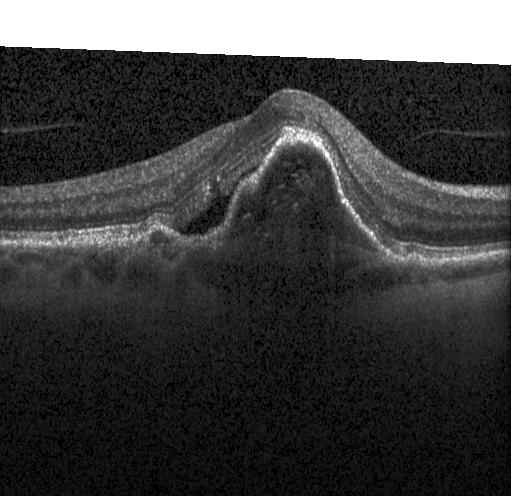

A choroidal neovascular membrane.